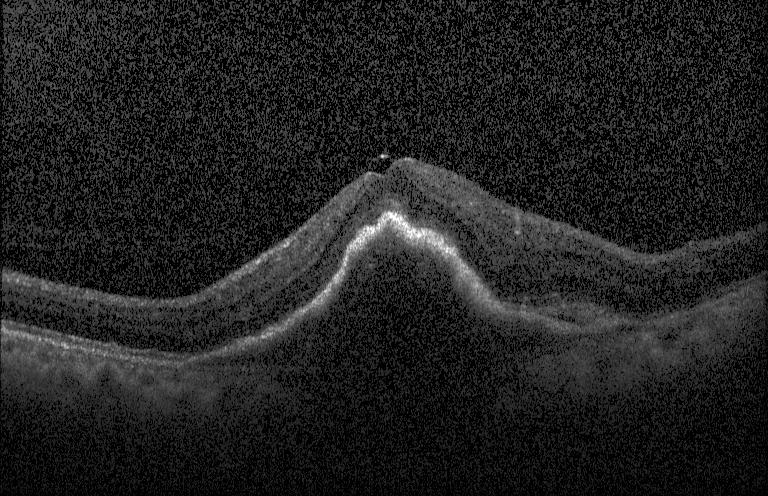 Optical coherence tomography scan.
The scan shows CNV.